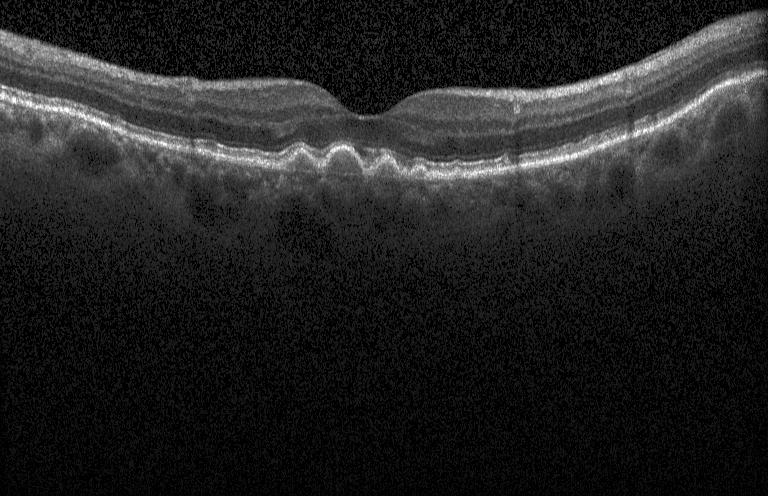
Heidelberg Spectralis · macular scan · optical coherence tomography scan · SD-OCT. OCT finding: drusen.